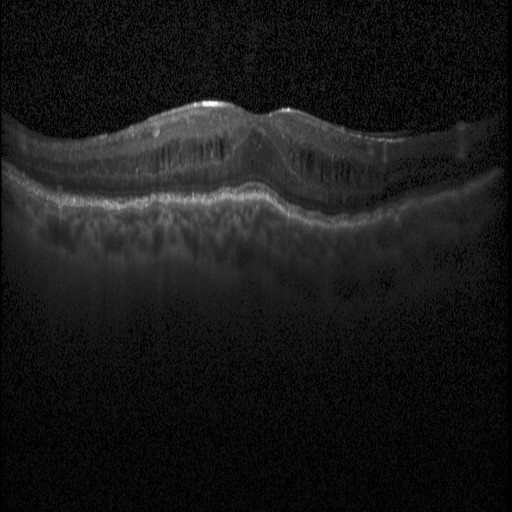

Optical coherence tomography B-scan, macular scan, spectral-domain OCT, instrument: Heidelberg Spectralis — This B-scan demonstrates diabetic macular edema.